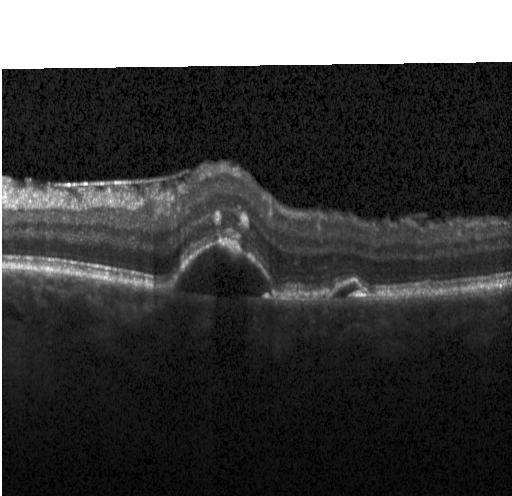 Diagnosis: choroidal neovascularization.